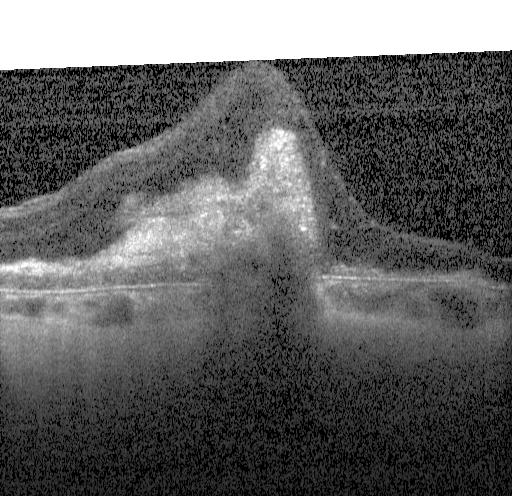
Spectral-domain OCT, OCT B-scan — Finding: choroidal neovascularization.